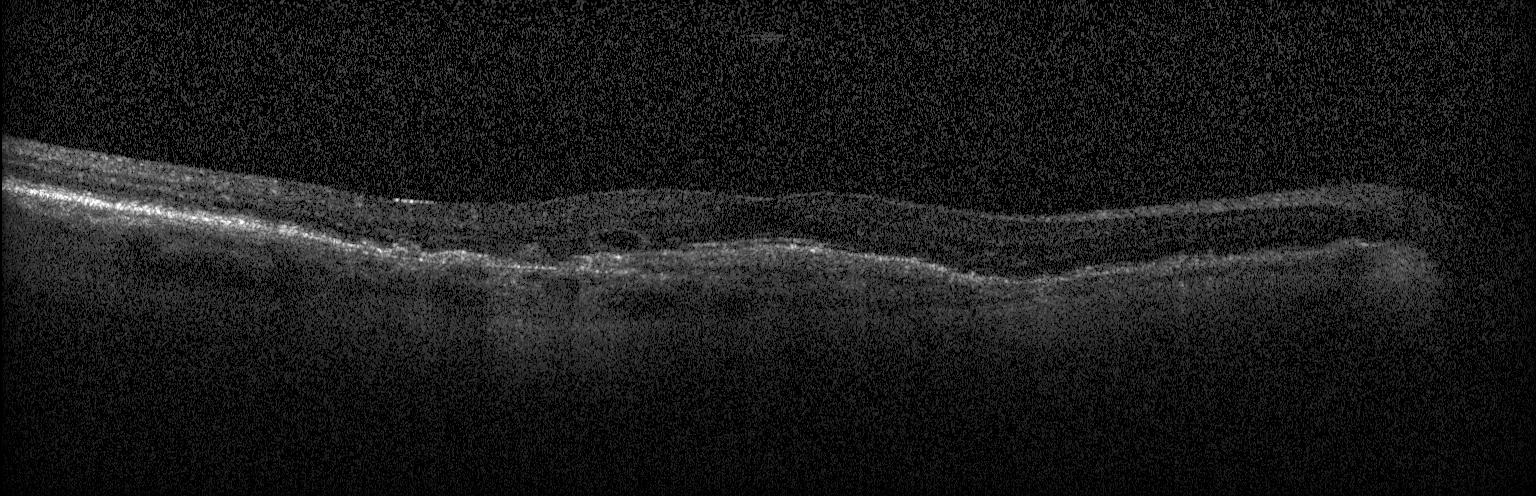

OCT B-scan.
This B-scan demonstrates a choroidal neovascular membrane.